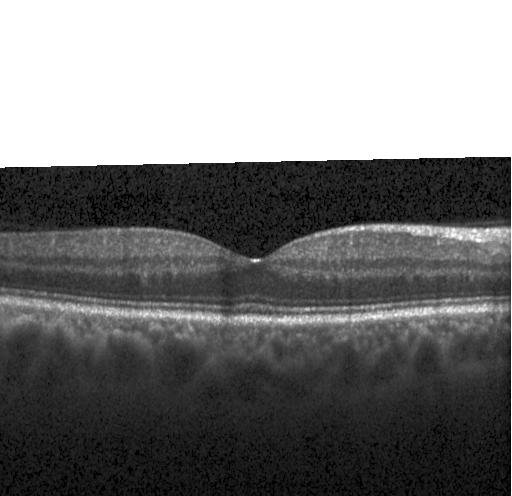
Optical coherence tomography scan, Heidelberg Spectralis OCT system — Assessment: no CNV, DME, or drusen.